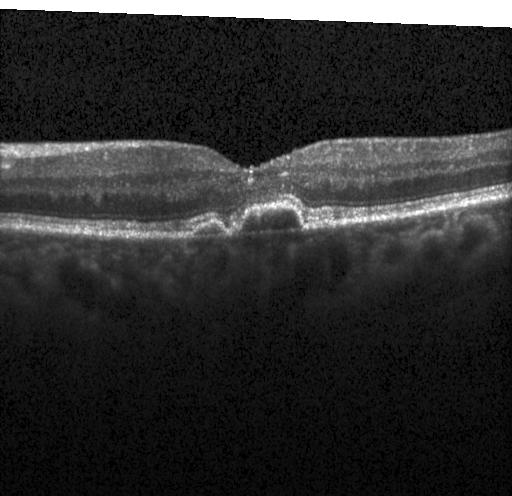 Fovea-centered; optical coherence tomography scan; Heidelberg Spectralis; spectral-domain optical coherence tomography
Impression: choroidal neovascularization.